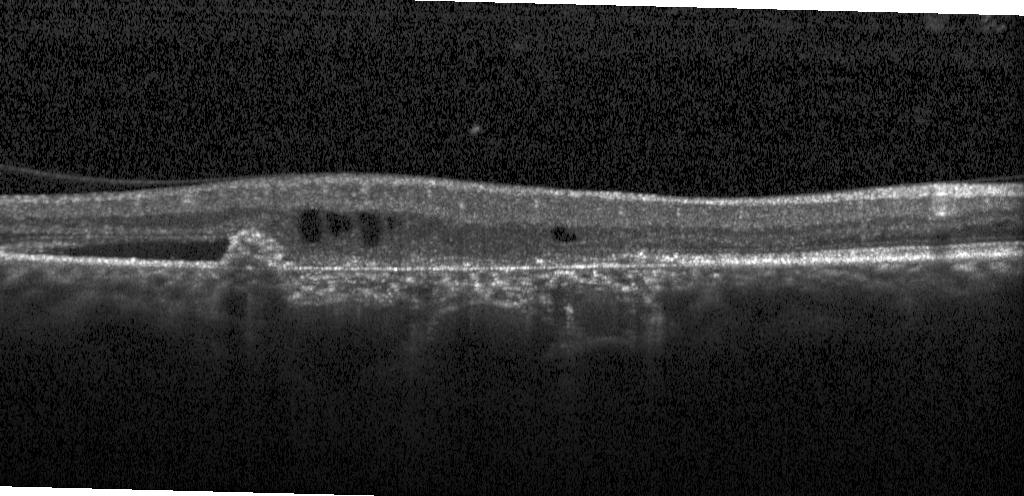 Diagnosis: a choroidal neovascular membrane.